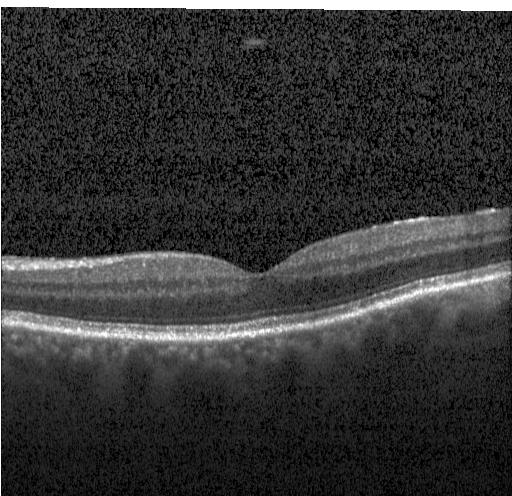
Diagnosis: no CNV, DME, or drusen.